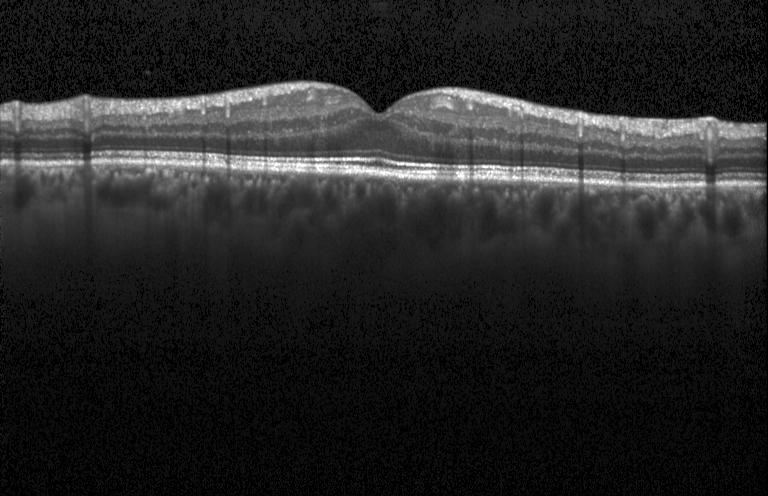 Centered on the fovea · optical coherence tomography B-scan · Heidelberg Spectralis OCT system. Assessment: neither choroidal neovascularization, diabetic macular edema, nor drusen.